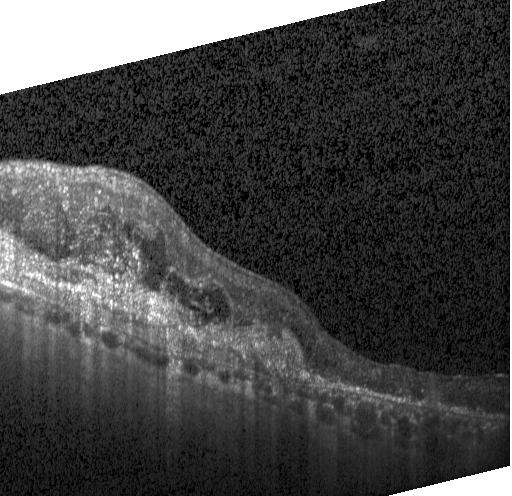
OCT line scan. Spectral-domain OCT.
Diagnosis: CNV.